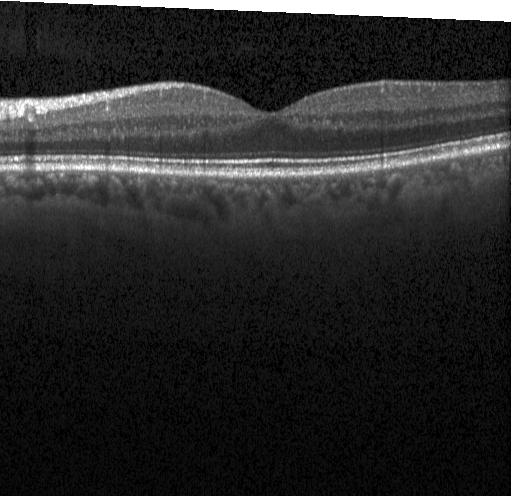 Retinal OCT cross-section — Diagnosis: no CNV, DME, or drusen.